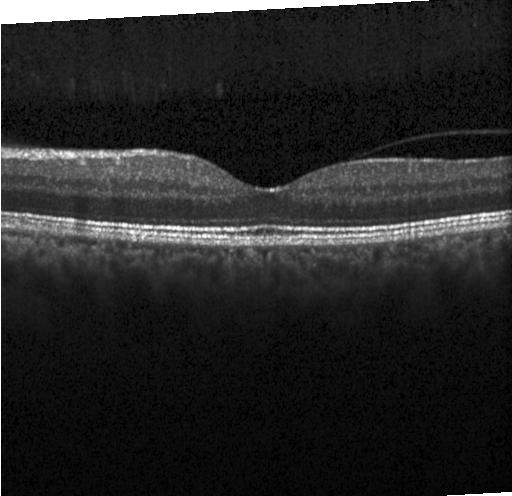 Fovea-centered. Optical coherence tomography B-scan.
Diagnosis: no evidence of choroidal neovascularization, diabetic macular edema, or drusen.